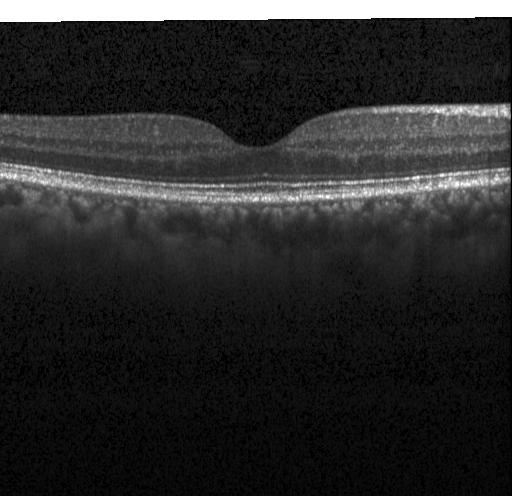 Retinal OCT cross-section — OCT finding: neither choroidal neovascularization, diabetic macular edema, nor drusen.